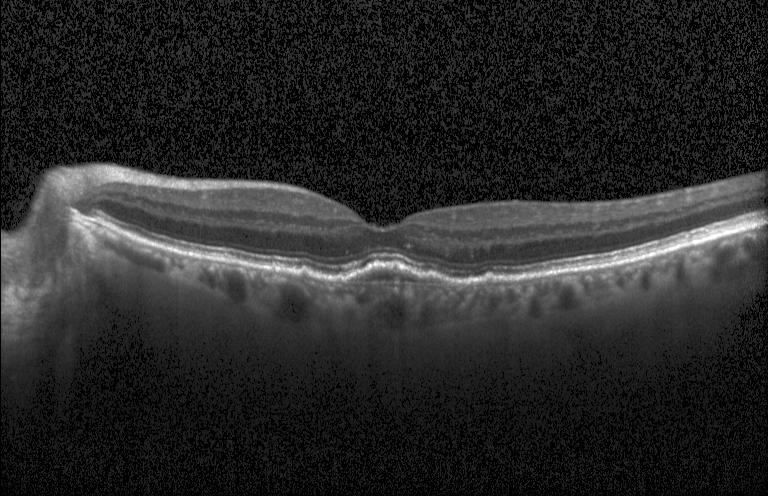
Spectral-domain OCT · Heidelberg Spectralis · OCT line scan · centered on the fovea.
Finding: choroidal neovascularization.